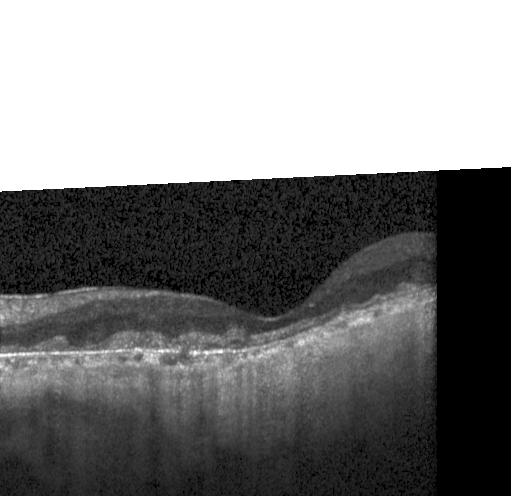
Instrument: Heidelberg Spectralis; retinal OCT B-scan; through the macula; SD-OCT. OCT finding: a choroidal neovascular membrane.